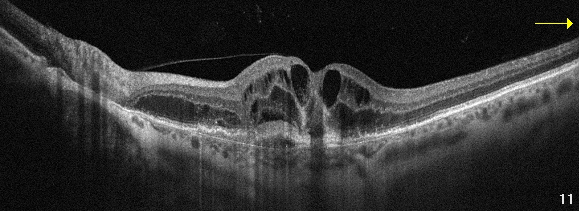

Macular OCT: age-related macular degeneration.